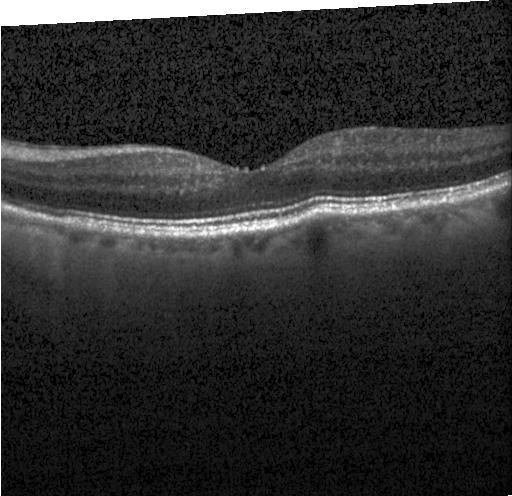 Retinal OCT B-scan — Multiple drusen.